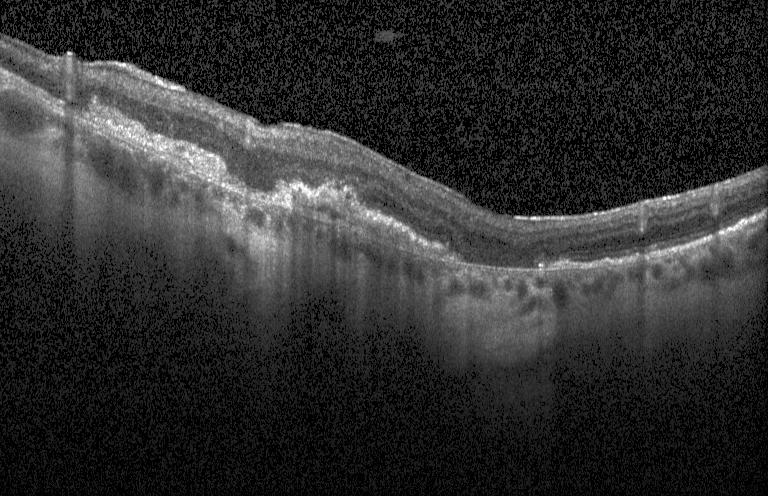 Spectral-domain OCT B-scan: a choroidal neovascular membrane.